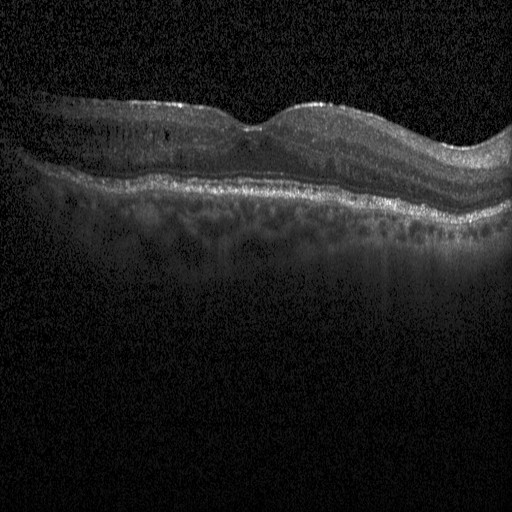
Macular OCT demonstrating DME.